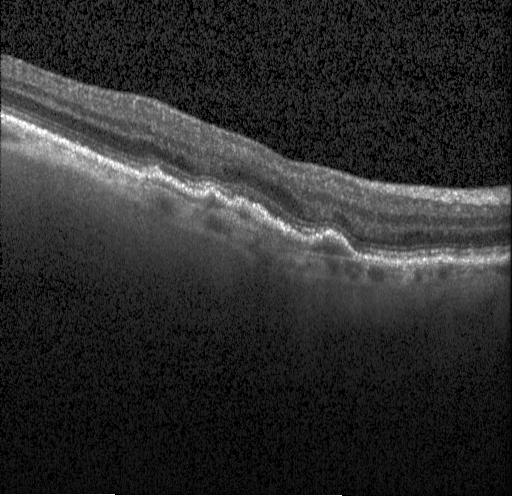 Heidelberg Spectralis OCT system, SD-OCT, OCT line scan, horizontal scan through the fovea.
Dx: a choroidal neovascular membrane.